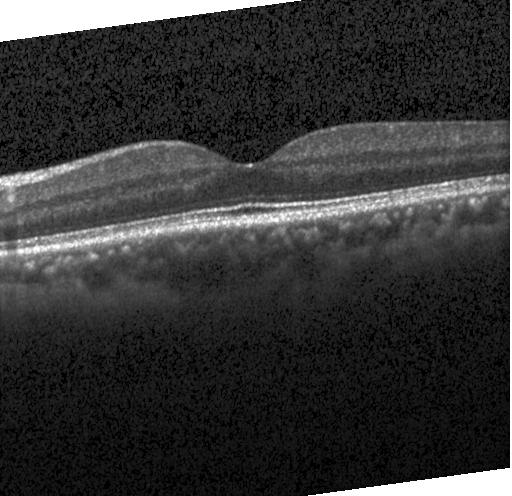
Diagnosis: no CNV, no DME, and no drusen.